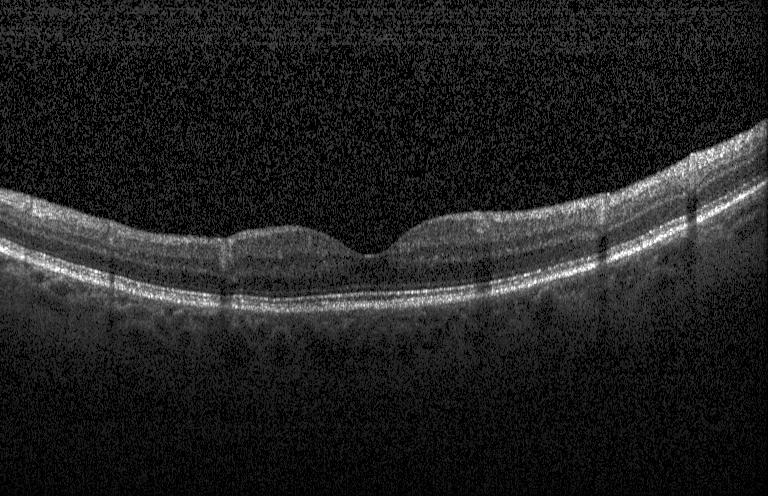

OCT B-scan showing no choroidal neovascularization, no diabetic macular edema, and no drusen.